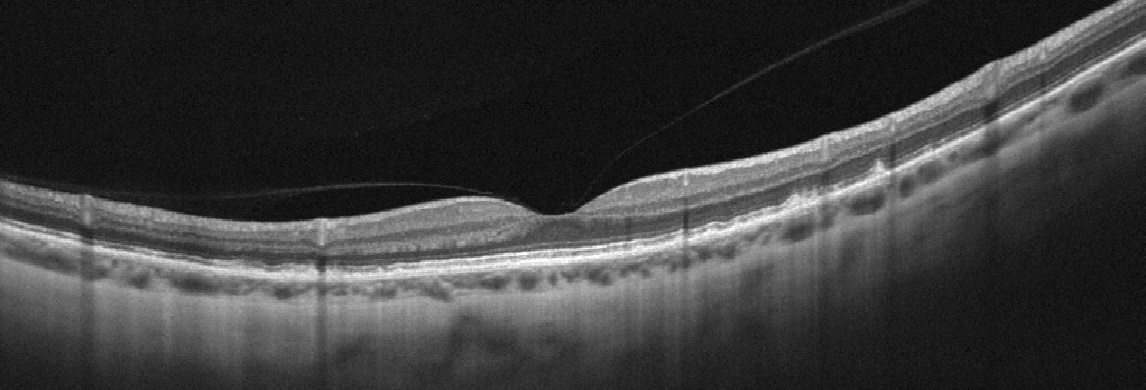

Through the macula; retinal OCT cross-section. The scan shows age-related macular degeneration.